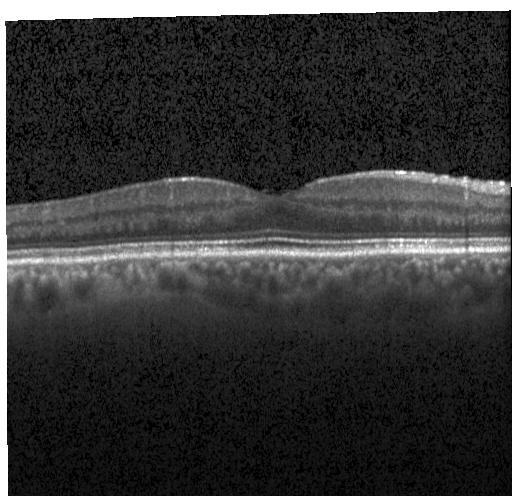
Finding: no evidence of CNV, DME, or drusen.